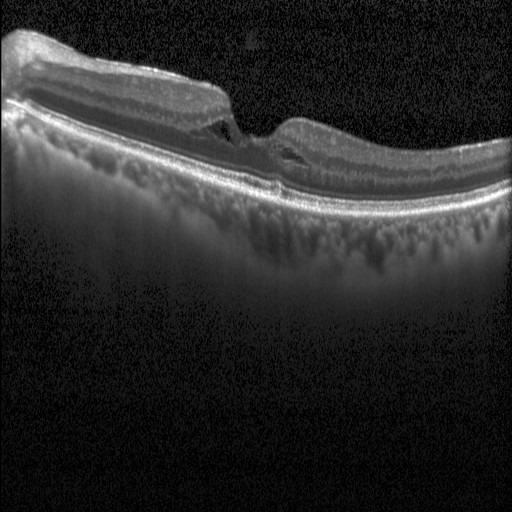

Optical coherence tomography scan, through the macula, instrument: Heidelberg Spectralis, spectral-domain optical coherence tomography — DME.